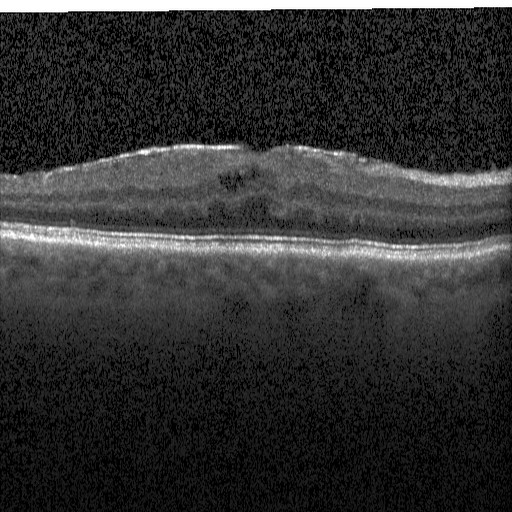

Retinal OCT cross-section showing DME.